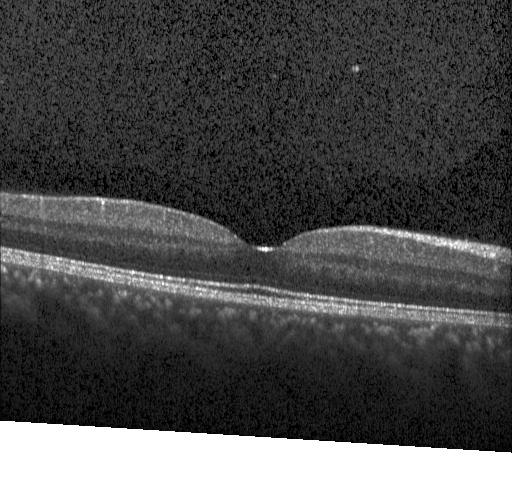

Optical coherence tomography B-scan · Heidelberg Spectralis OCT system.
Diagnosis: no choroidal neovascularization, diabetic macular edema, or drusen.